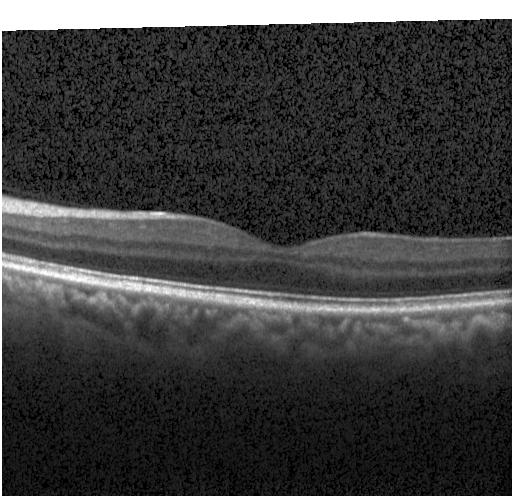
The scan shows neither choroidal neovascularization, diabetic macular edema, nor drusen.